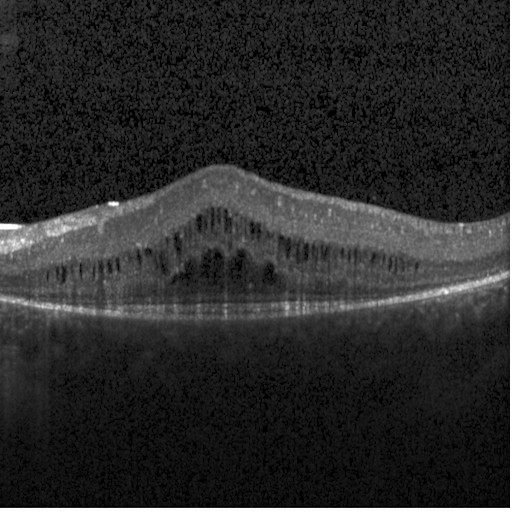

OCT finding: diabetic macular edema.